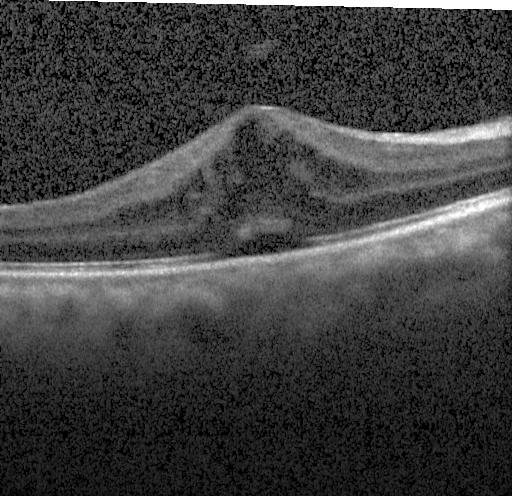
Optical coherence tomography B-scan
This B-scan demonstrates diabetic macular edema.